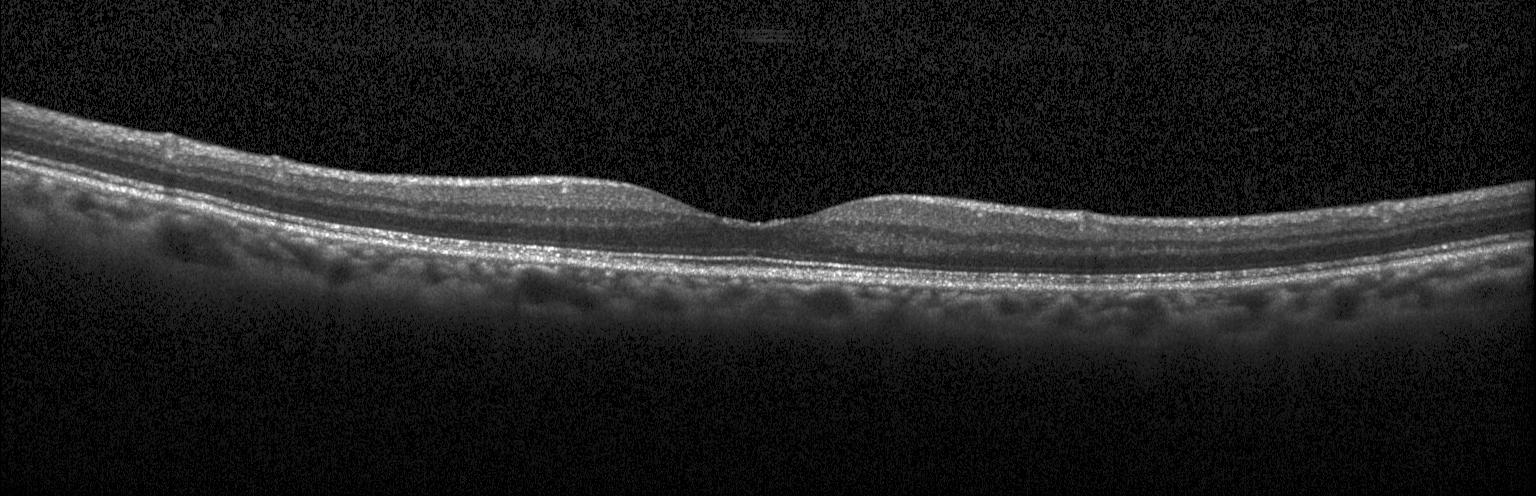
Heidelberg Spectralis, spectral-domain OCT, retinal OCT cross-section — Assessment: no CNV, DME, or drusen.